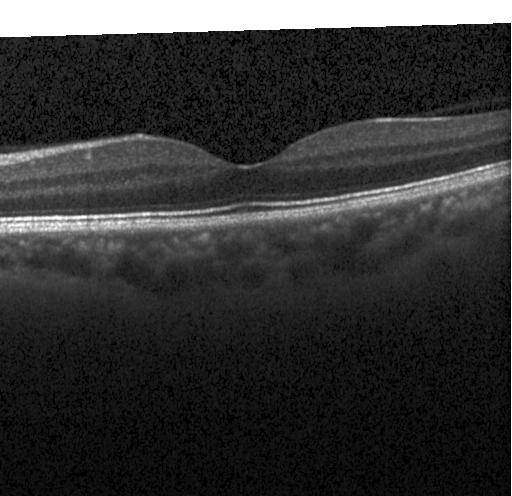

Optical coherence tomography B-scan.
Finding: neither choroidal neovascularization, diabetic macular edema, nor drusen.